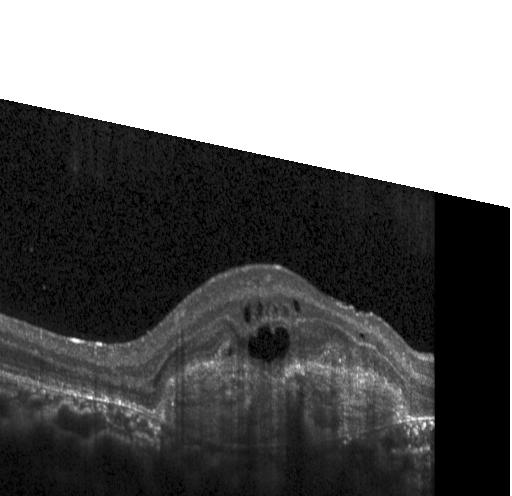 OCT B-scan. Macular OCT: a choroidal neovascular membrane.